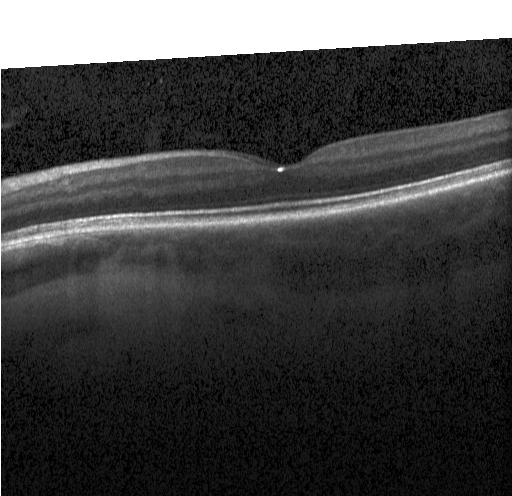

Optical coherence tomography B-scan; spectral-domain optical coherence tomography; Heidelberg Spectralis; centered on the fovea — Diagnosis: neither CNV, DME, nor drusen.